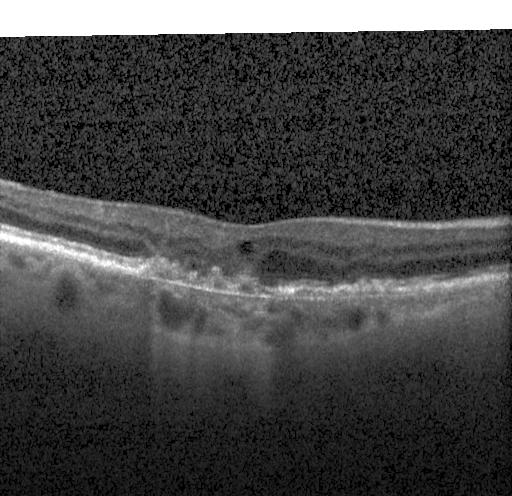 Spectral-domain optical coherence tomography · Heidelberg Spectralis · optical coherence tomography B-scan. Diagnosis: choroidal neovascularization (CNV).